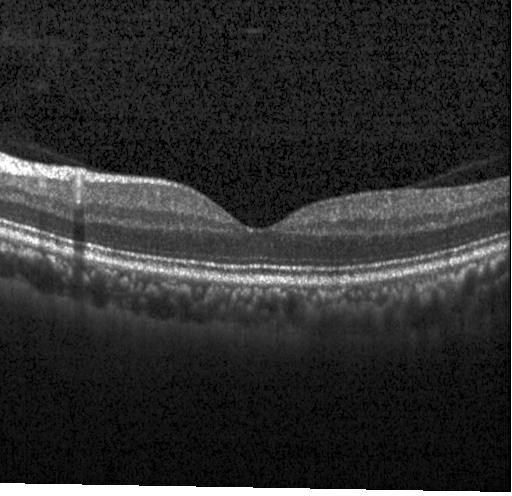

Heidelberg Spectralis. Spectral-domain OCT. OCT B-scan. Macular OCT: neither CNV, DME, nor drusen.